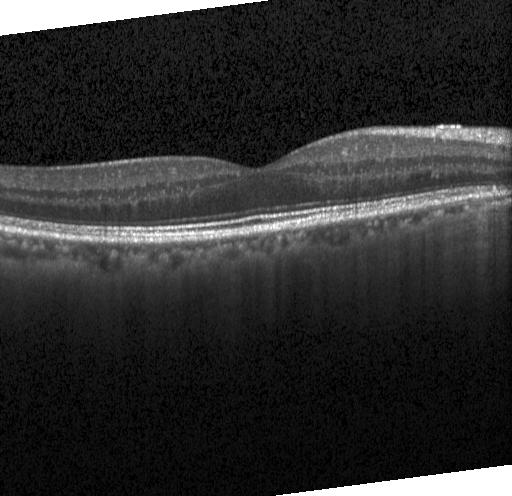

Dx: neither choroidal neovascularization, diabetic macular edema, nor drusen.